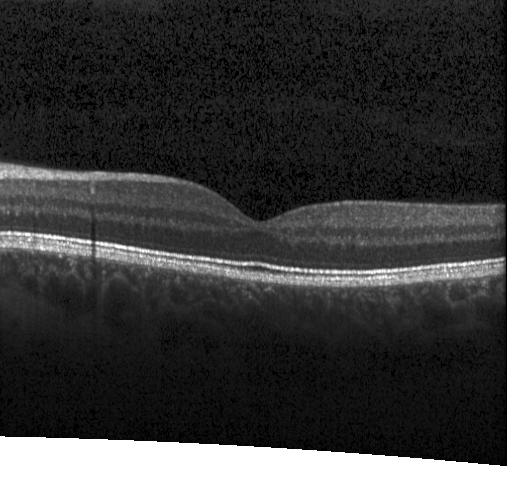 Retinal OCT cross-section, macular scan, spectral-domain OCT, instrument: Heidelberg Spectralis. The scan shows no CNV, DME, or drusen.